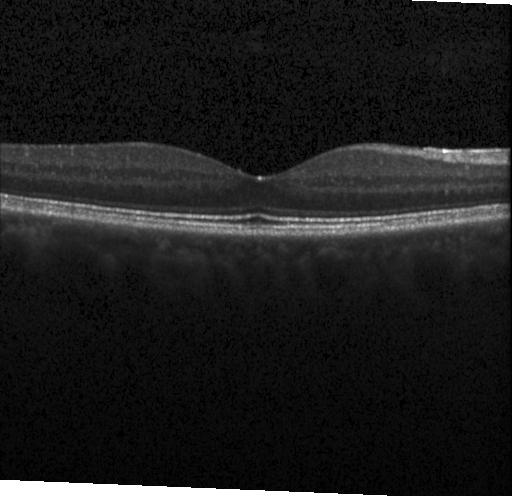
Optical coherence tomography scan.
Macular OCT: no evidence of CNV, DME, or drusen.